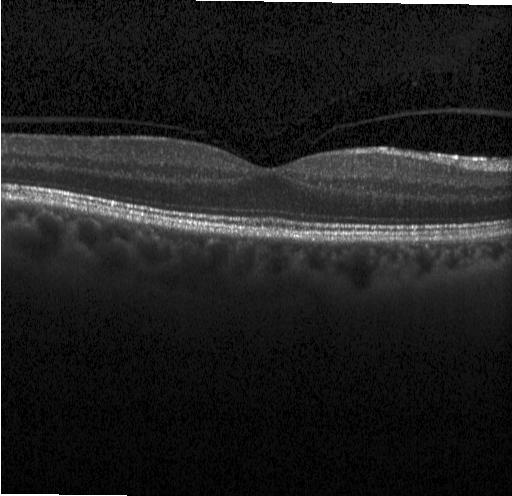

Dx: neither CNV, DME, nor drusen.